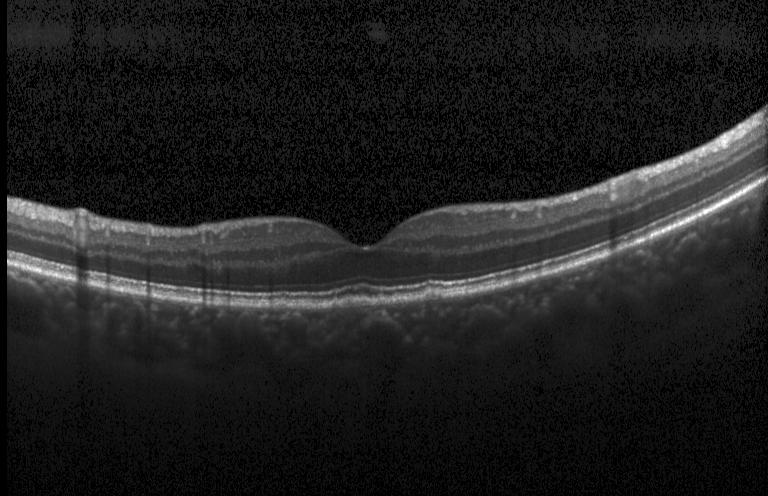

This B-scan demonstrates sub-RPE drusenoid deposits.